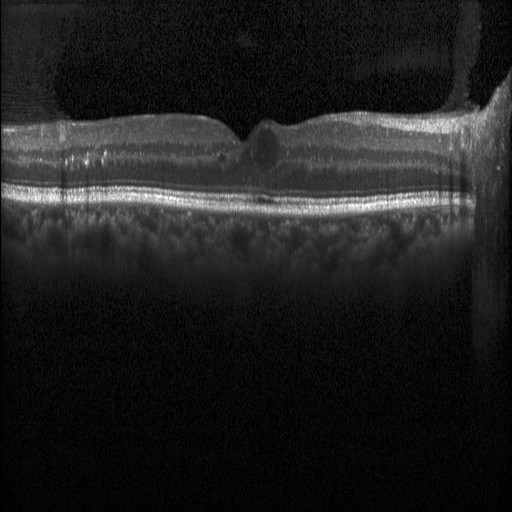
Fovea-centered, instrument: Heidelberg Spectralis, OCT B-scan. Finding: DME.